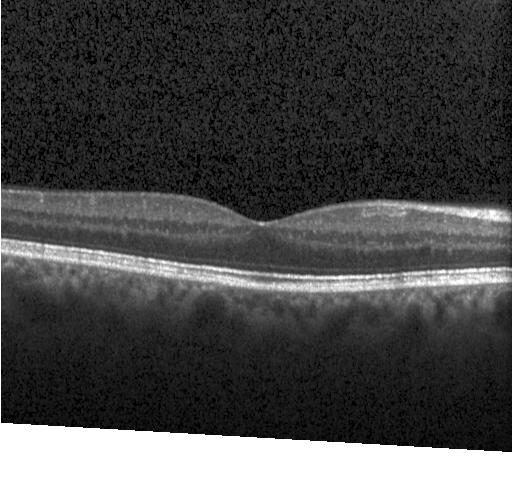 Horizontal scan through the fovea. Retinal OCT B-scan. Acquired on a Heidelberg Spectralis — Impression: no CNV, DME, or drusen.